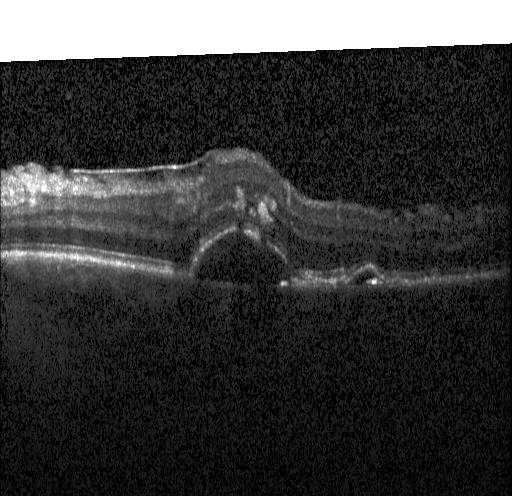
Macular OCT: a choroidal neovascular membrane.